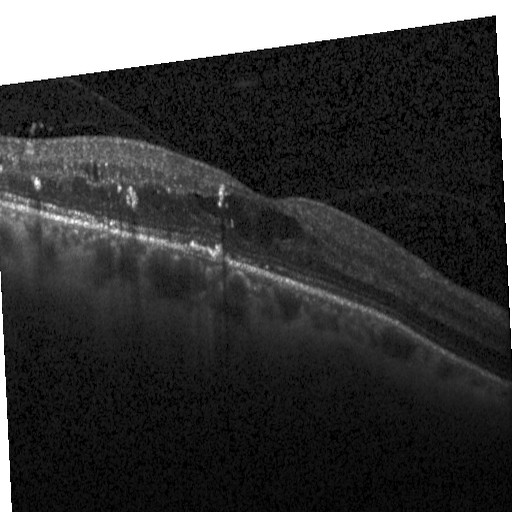

SD-OCT, Heidelberg Spectralis OCT system, through the macula, retinal OCT B-scan.
This B-scan demonstrates diabetic macular edema.